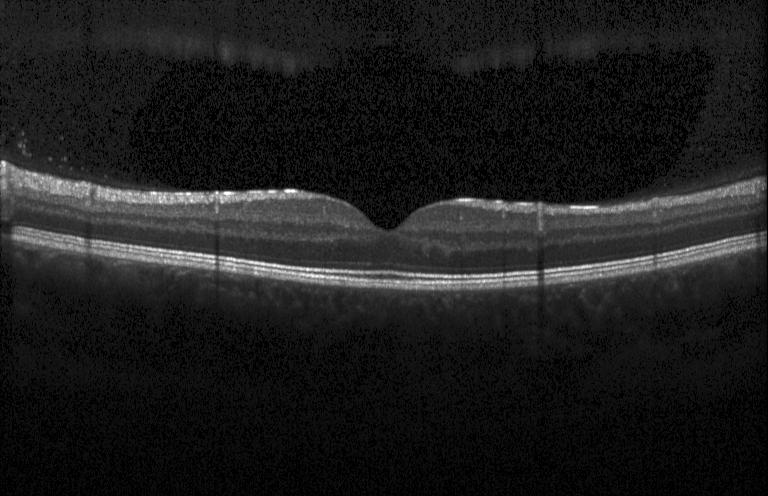
OCT finding: neither choroidal neovascularization, diabetic macular edema, nor drusen.